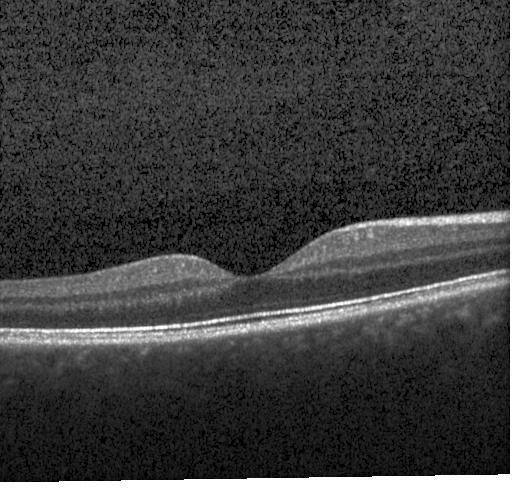
Optical coherence tomography scan; Heidelberg Spectralis; macular scan. Diagnosis: no evidence of choroidal neovascularization, diabetic macular edema, or drusen.